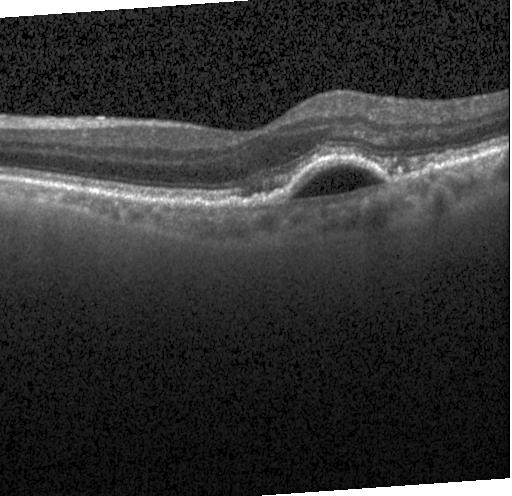 SD-OCT · optical coherence tomography scan
Impression: a choroidal neovascular membrane.